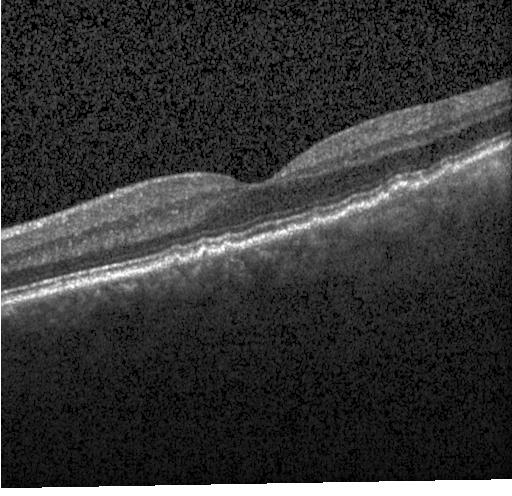
Assessment: sub-RPE drusenoid deposits.